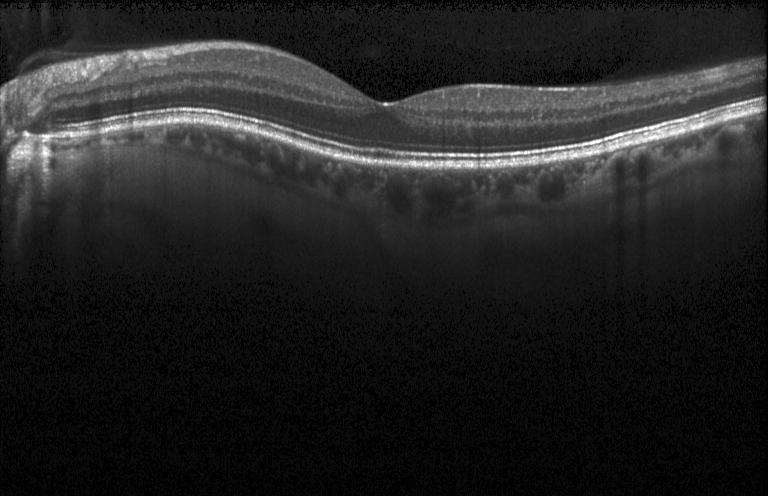

Optical coherence tomography B-scan.
Diagnosis: neither choroidal neovascularization, diabetic macular edema, nor drusen.